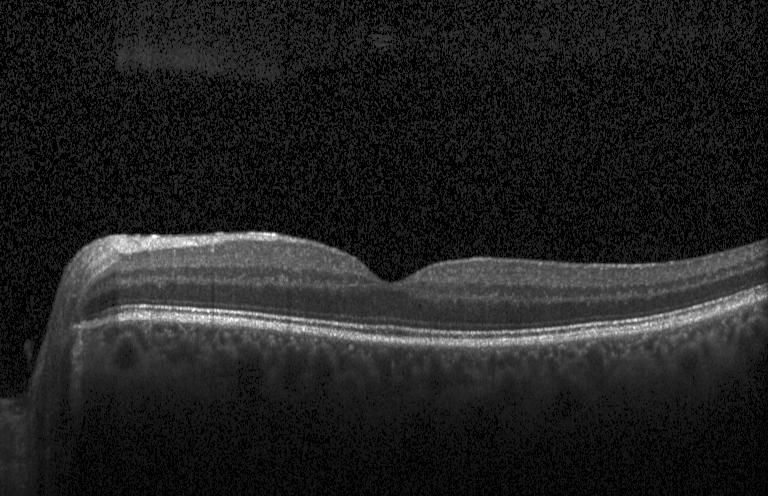 Macular OCT: neither choroidal neovascularization, diabetic macular edema, nor drusen.